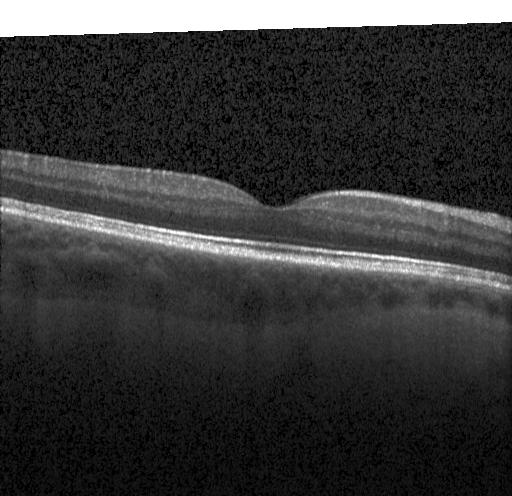
Fovea-centered; OCT B-scan; Heidelberg Spectralis OCT system — Diagnosis: no evidence of CNV, DME, or drusen.